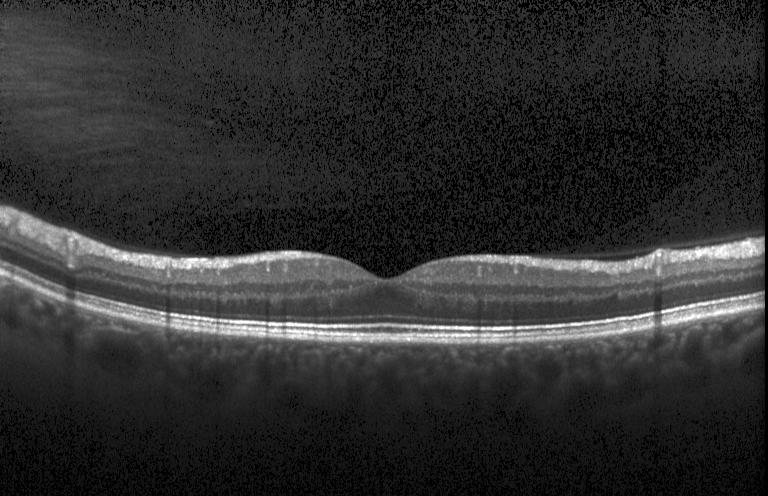
OCT line scan. Impression: neither choroidal neovascularization, diabetic macular edema, nor drusen.